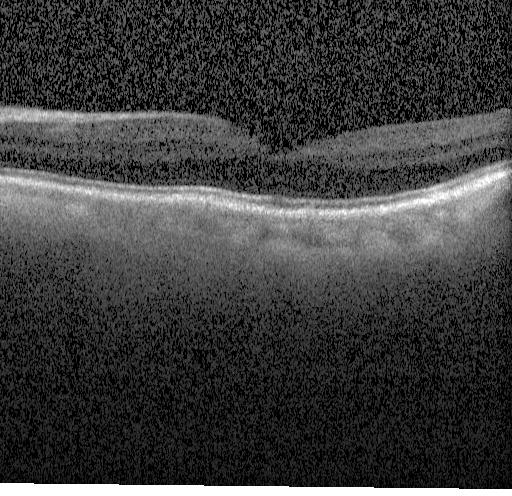

Retinal OCT B-scan.
Impression: neither choroidal neovascularization, diabetic macular edema, nor drusen.